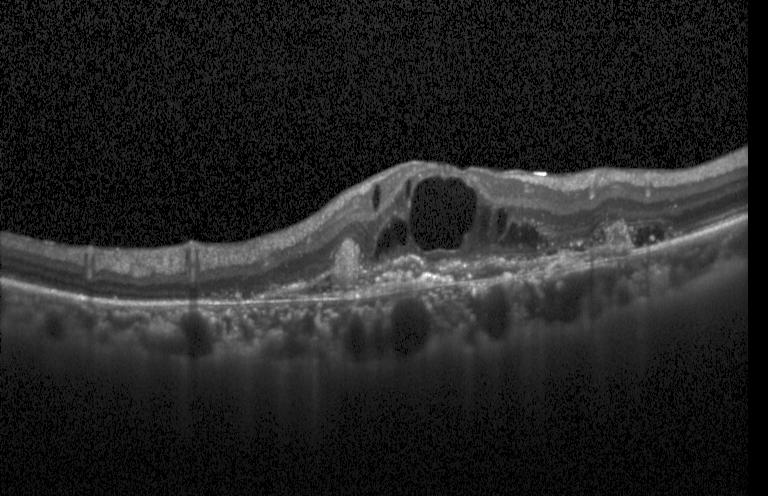

Impression: CNV.